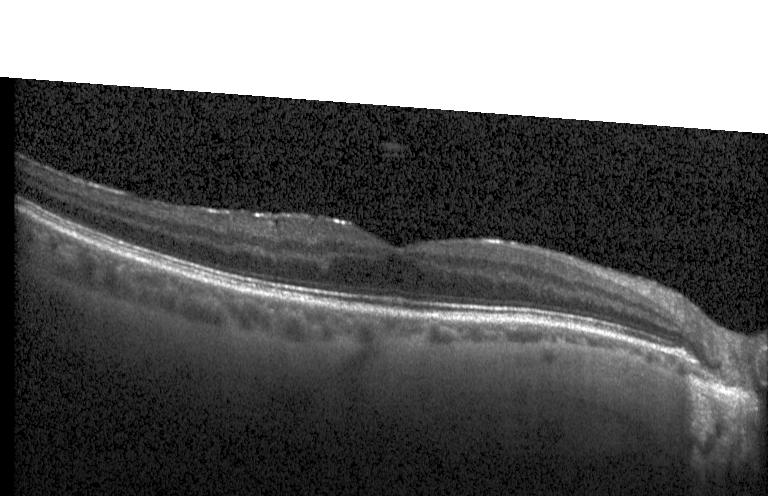

OCT line scan; spectral-domain OCT. Diagnosis: no evidence of choroidal neovascularization, diabetic macular edema, or drusen.